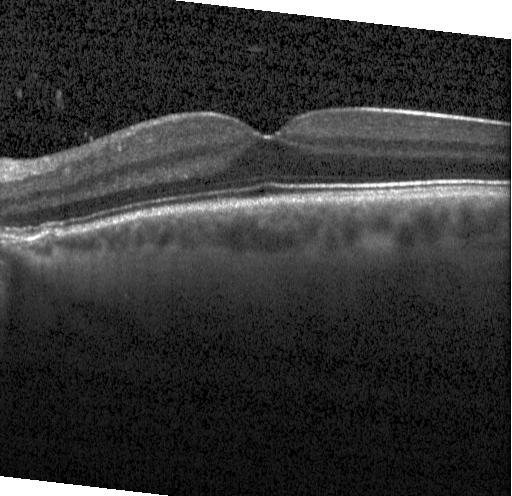
Macular OCT: drusen.